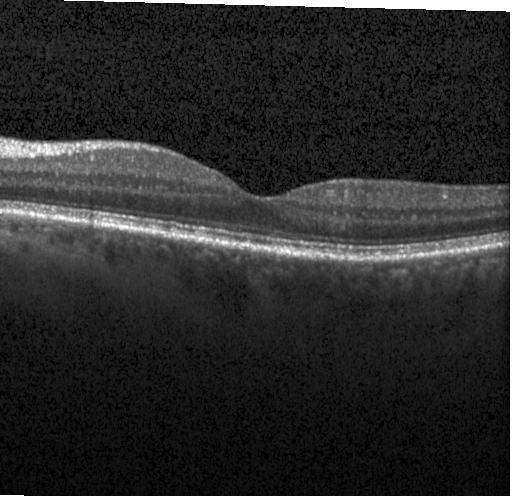

Macular OCT: neither choroidal neovascularization, diabetic macular edema, nor drusen.